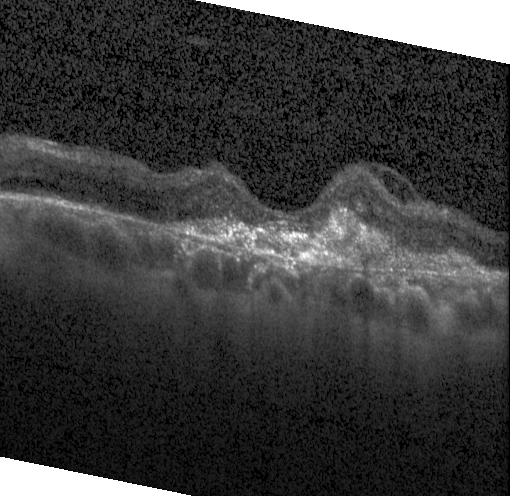 Choroidal neovascularization.